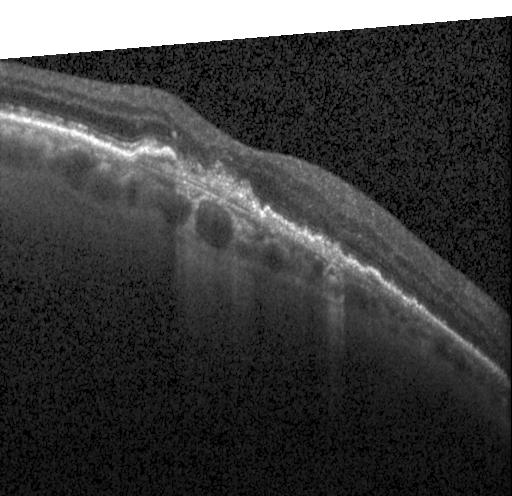 Centered on the fovea · Heidelberg Spectralis · spectral-domain optical coherence tomography · retinal OCT cross-section
Impression: choroidal neovascularization (CNV).